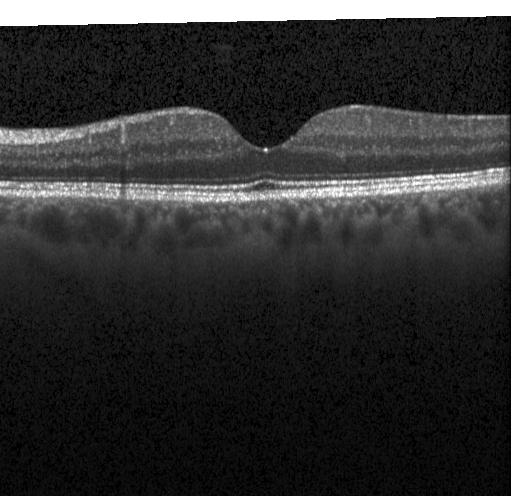
OCT B-scan, spectral-domain optical coherence tomography.
Dx: neither choroidal neovascularization, diabetic macular edema, nor drusen.